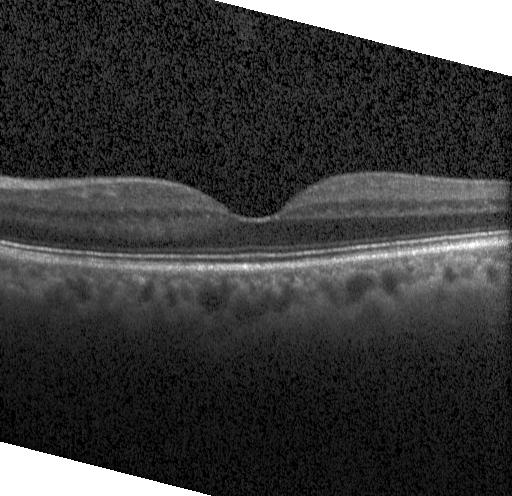

Heidelberg Spectralis, horizontal scan through the fovea, OCT B-scan, spectral-domain optical coherence tomography
This B-scan demonstrates no evidence of choroidal neovascularization, diabetic macular edema, or drusen.